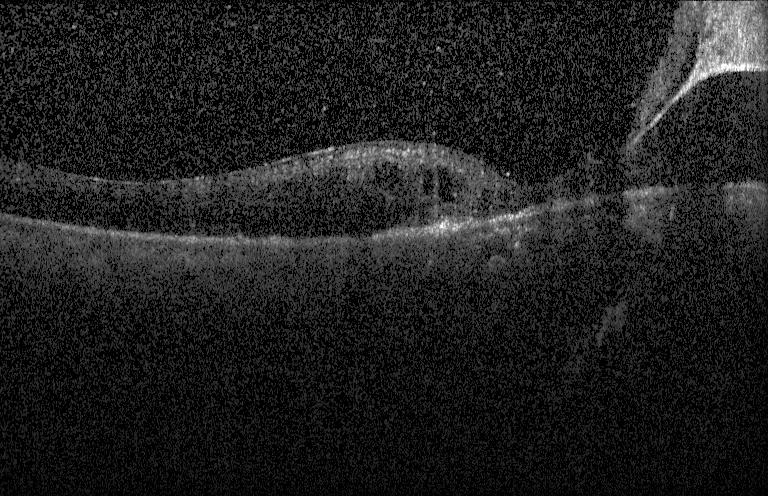
OCT scan showing diabetic macular edema.